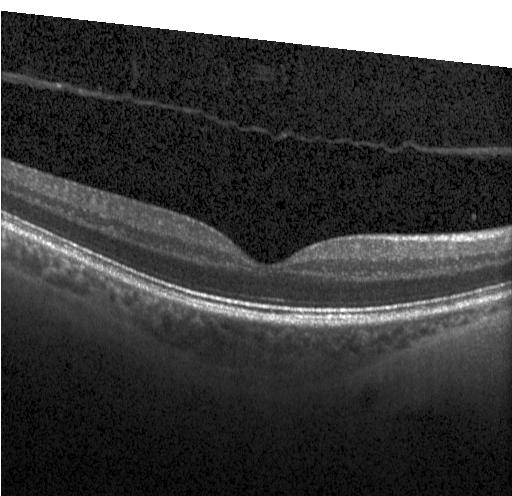
Retinal OCT cross-section
Diagnosis: neither choroidal neovascularization, diabetic macular edema, nor drusen.